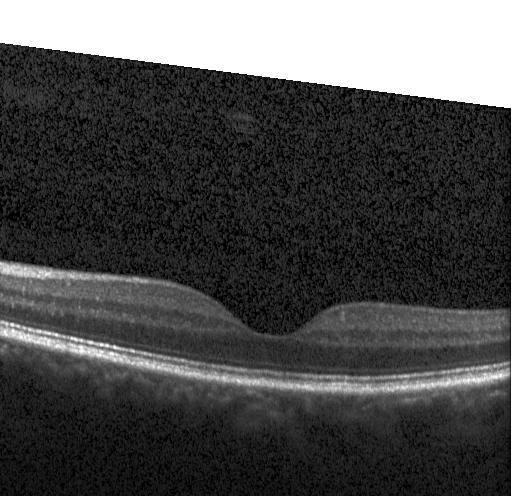

Diagnosis: neither choroidal neovascularization, diabetic macular edema, nor drusen.